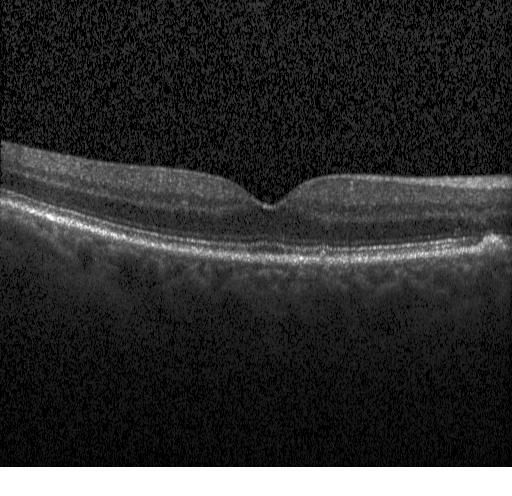
Retinal OCT cross-section; spectral-domain optical coherence tomography.
Impression: no CNV, no DME, and no drusen.